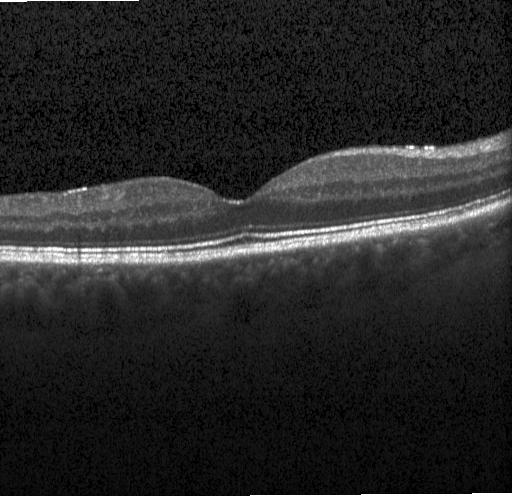

Macular scan, spectral-domain optical coherence tomography, optical coherence tomography B-scan — Finding: no CNV, DME, or drusen.